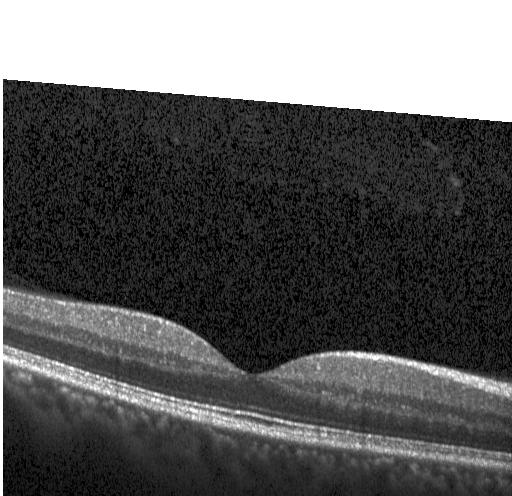

Spectral-domain optical coherence tomography, acquired on a Heidelberg Spectralis, centered on the fovea, retinal OCT B-scan
Macular OCT: no choroidal neovascularization, diabetic macular edema, or drusen.